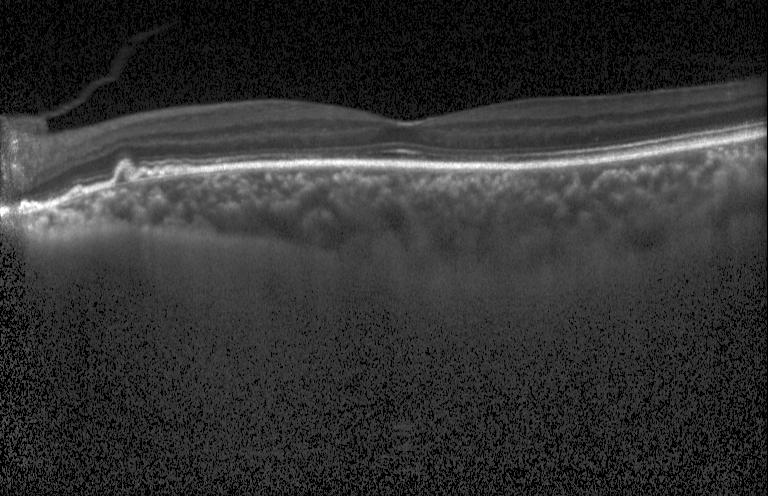

OCT line scan — Impression: sub-RPE drusenoid deposits.